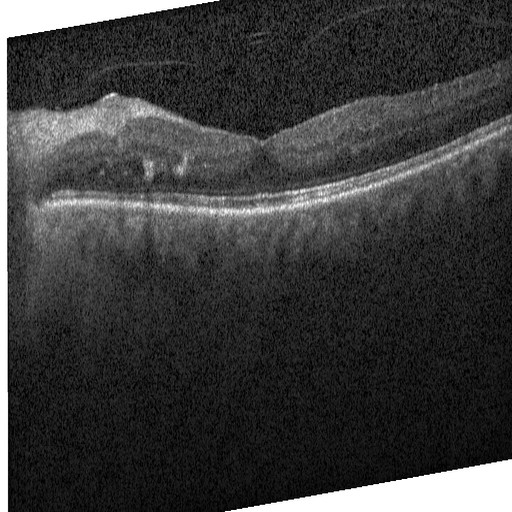

Retinal OCT B-scan. Finding: diabetic macular edema (DME).